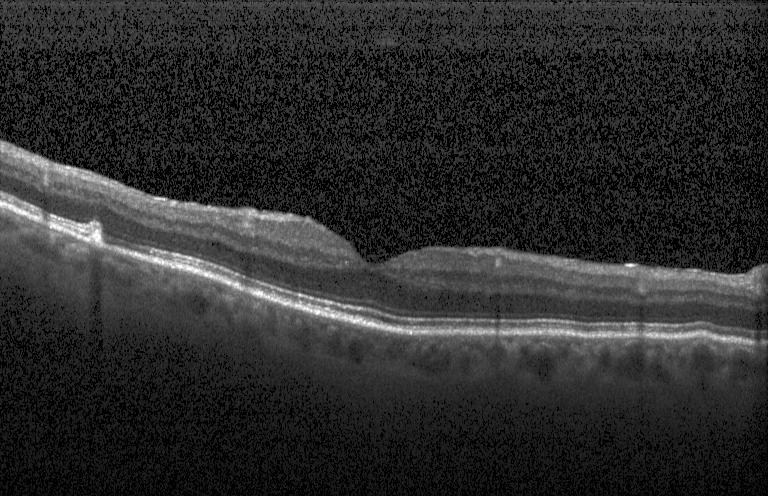

Optical coherence tomography scan · SD-OCT · acquired on a Heidelberg Spectralis.
Dx: sub-RPE drusenoid deposits.